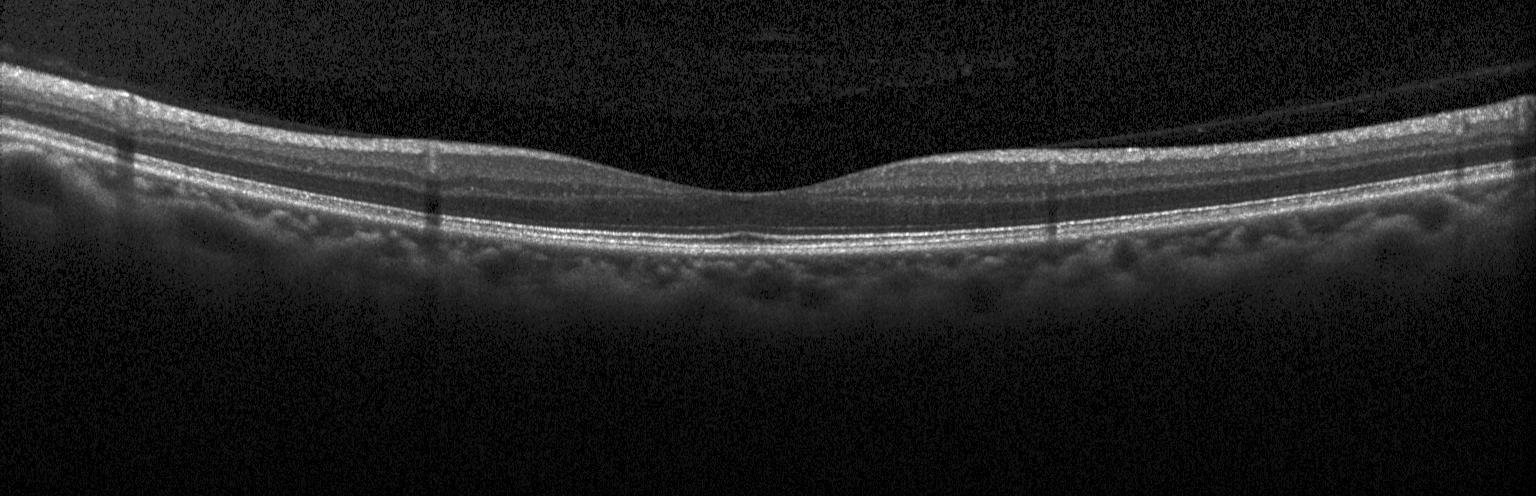
Retinal OCT cross-section showing neither CNV, DME, nor drusen.